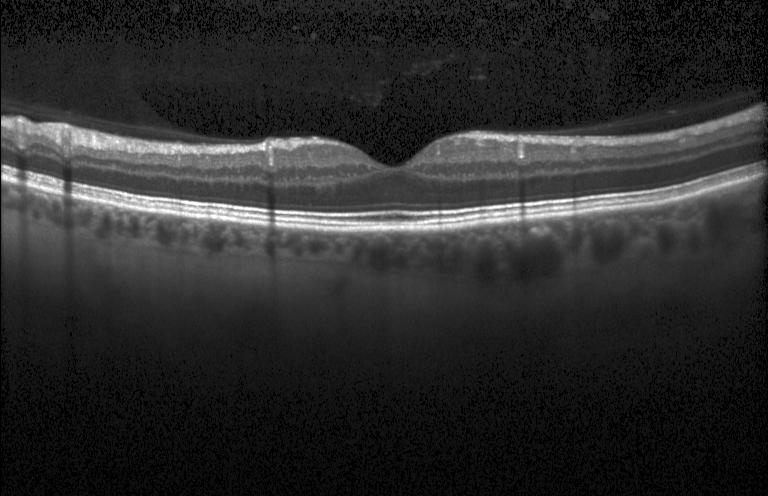 Optical coherence tomography scan. Dx: no choroidal neovascularization, diabetic macular edema, or drusen.